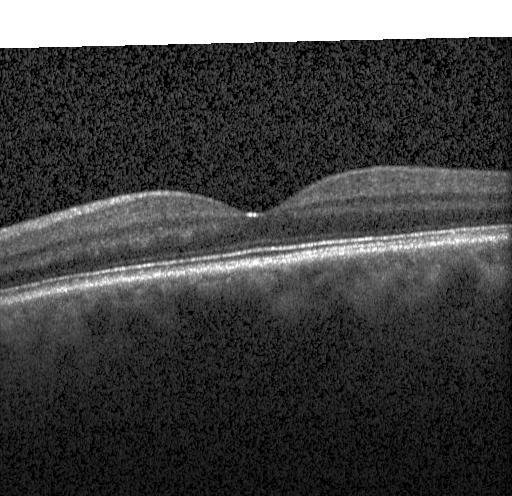 OCT scan showing neither choroidal neovascularization, diabetic macular edema, nor drusen.